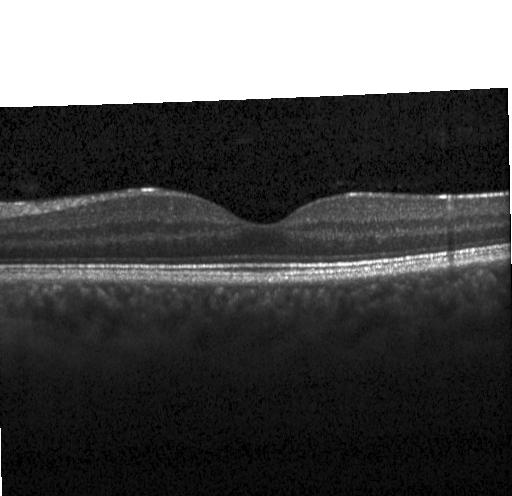 Retinal OCT cross-section. Diagnosis: neither CNV, DME, nor drusen.